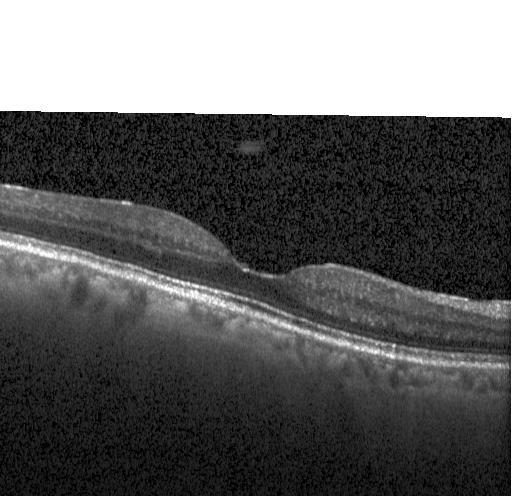
Through the macula · OCT B-scan — Finding: no evidence of choroidal neovascularization, diabetic macular edema, or drusen.